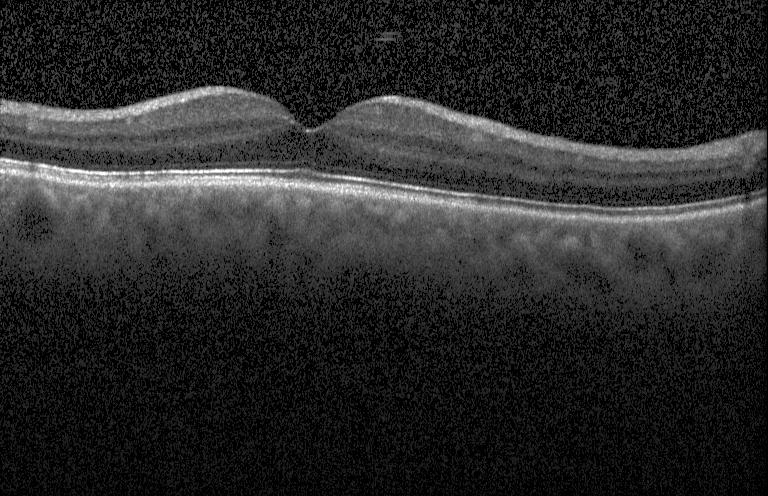
OCT finding: neither CNV, DME, nor drusen.